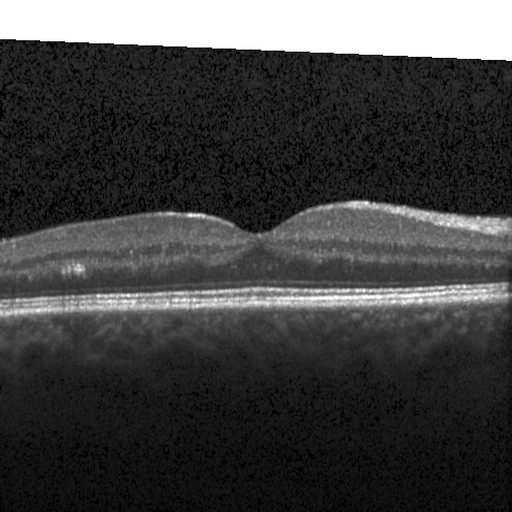 Spectral-domain optical coherence tomography, Heidelberg Spectralis OCT system, OCT B-scan. The scan shows DME.